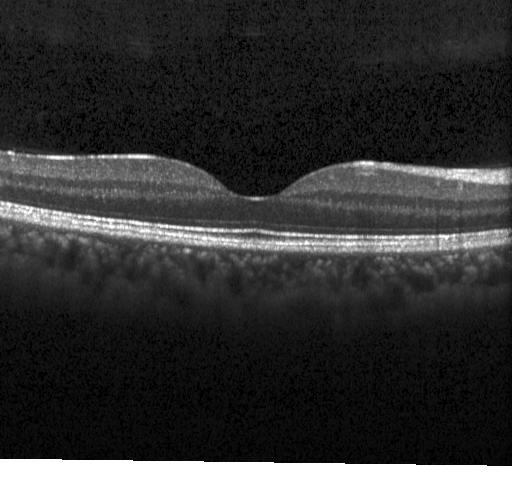
Heidelberg Spectralis OCT system, optical coherence tomography scan, spectral-domain OCT
This B-scan demonstrates neither choroidal neovascularization, diabetic macular edema, nor drusen.